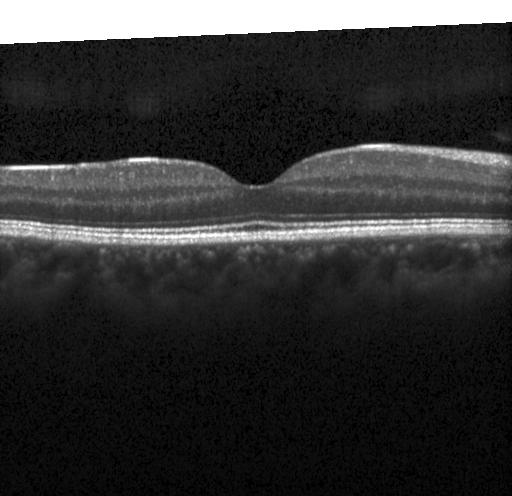 Spectral-domain OCT; fovea-centered; optical coherence tomography B-scan; instrument: Heidelberg Spectralis. Impression: no choroidal neovascularization, no diabetic macular edema, and no drusen.